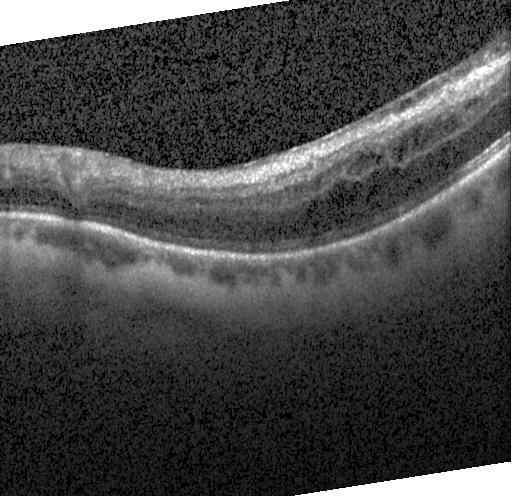

OCT B-scan — Finding: DME.